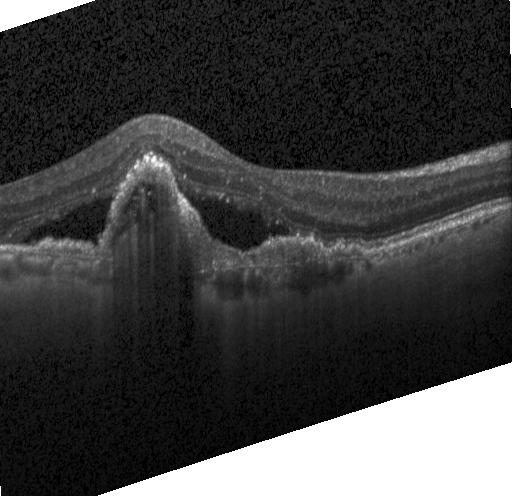

Diagnosis: choroidal neovascularization (CNV).